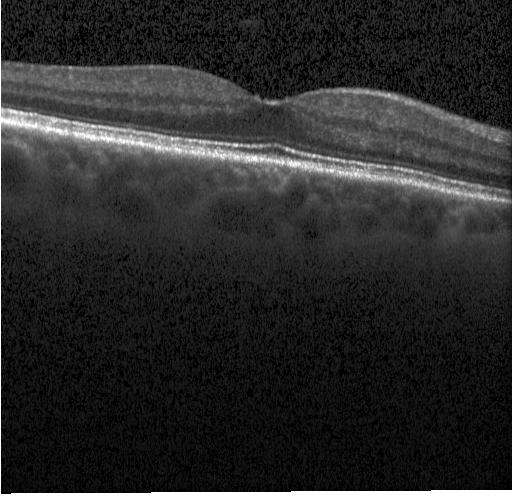
Through the macula; optical coherence tomography B-scan
Macular OCT: no evidence of choroidal neovascularization, diabetic macular edema, or drusen.